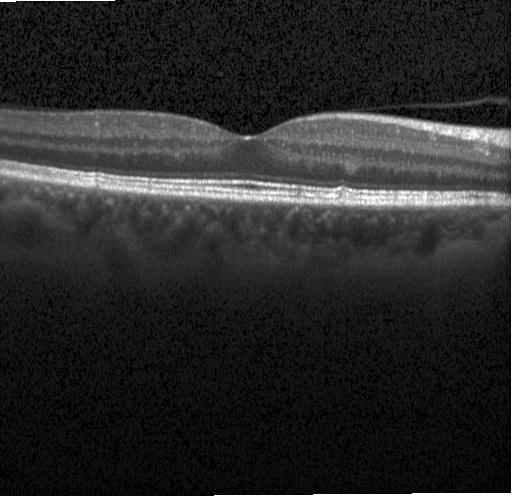

OCT B-scan. Finding: multiple drusen.